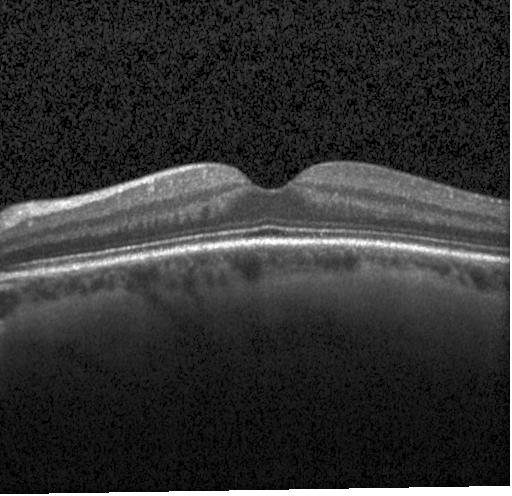
Instrument: Heidelberg Spectralis · spectral-domain optical coherence tomography · macular scan · retinal OCT cross-section. No evidence of choroidal neovascularization, diabetic macular edema, or drusen.